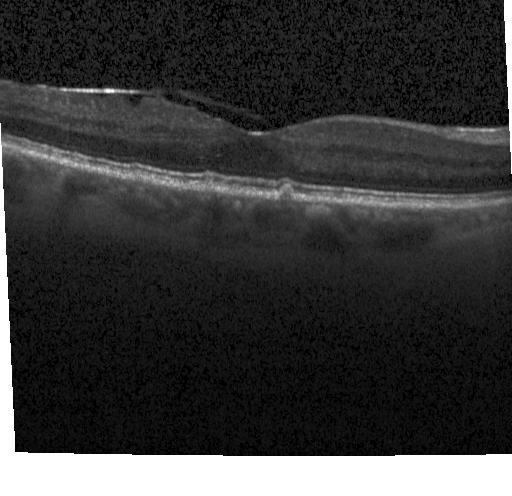

Retinal OCT B-scan. The scan shows sub-RPE drusenoid deposits.